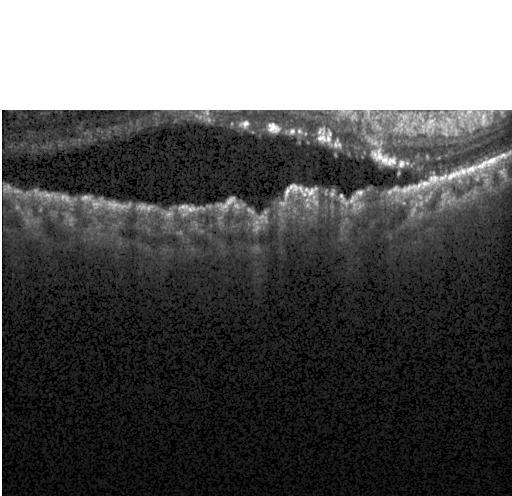 Assessment: a choroidal neovascular membrane.